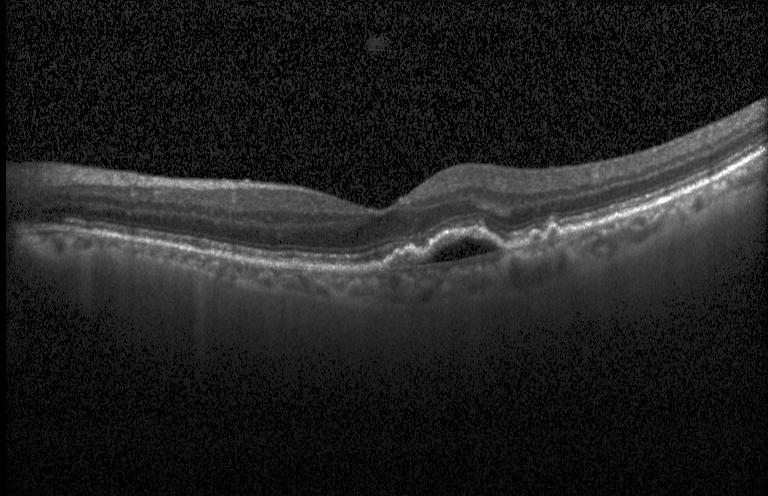
Dx: choroidal neovascularization (CNV).